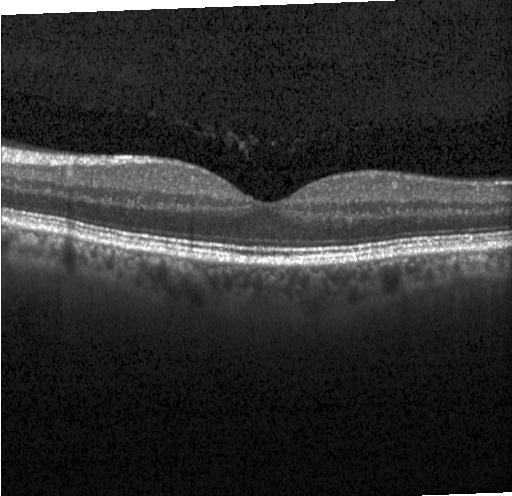

SD-OCT; centered on the fovea; OCT B-scan; Heidelberg Spectralis OCT system. Macular OCT: no evidence of CNV, DME, or drusen.